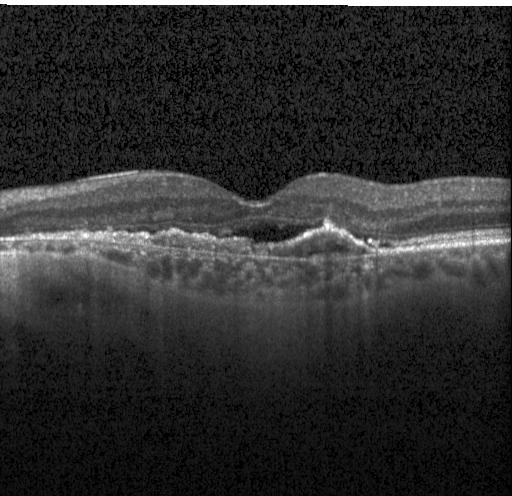 Fovea-centered · spectral-domain OCT · instrument: Heidelberg Spectralis · optical coherence tomography B-scan. Diagnosis: choroidal neovascularization.